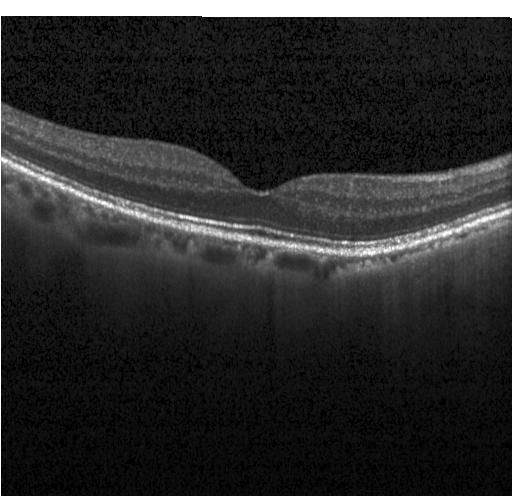 Impression: no choroidal neovascularization, no diabetic macular edema, and no drusen.